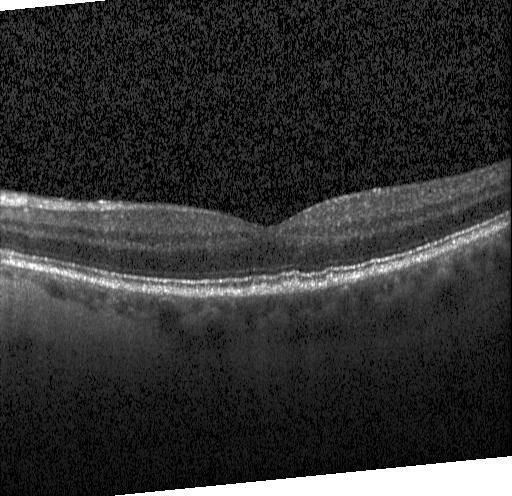

Retinal OCT cross-section.
Diagnosis: sub-RPE drusenoid deposits.